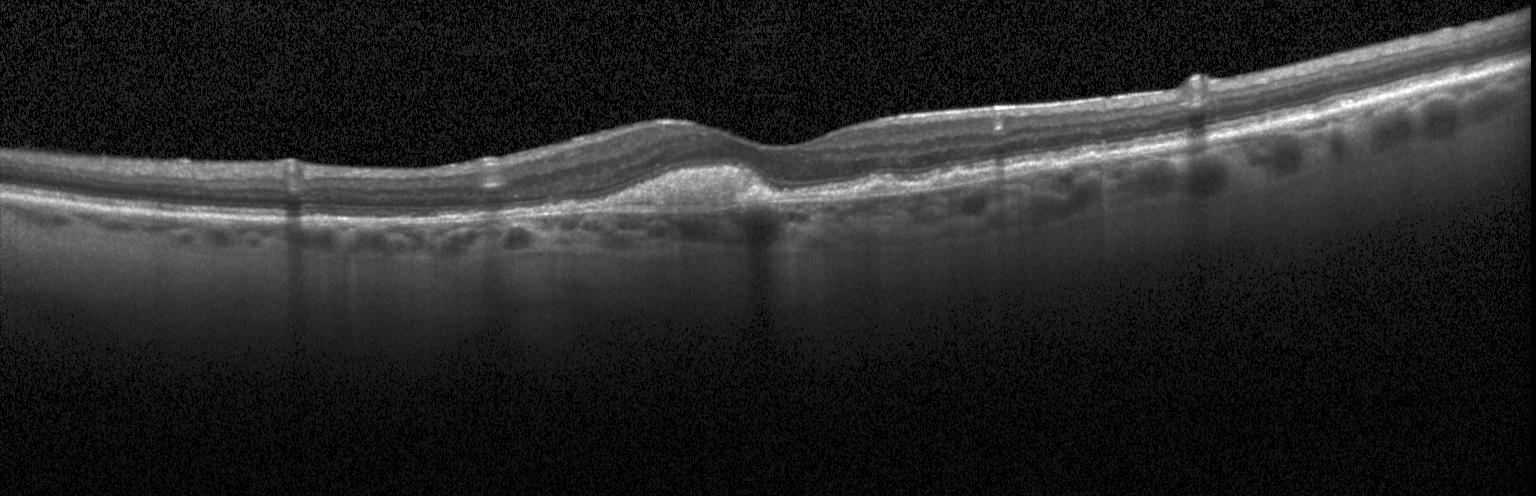

Retinal OCT cross-section — Impression: a choroidal neovascular membrane.